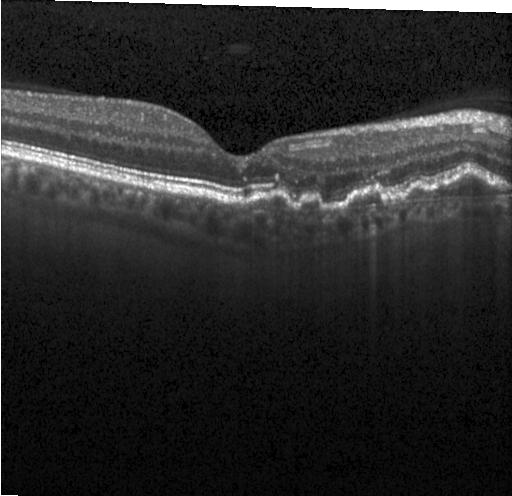

OCT B-scan. Impression: CNV.